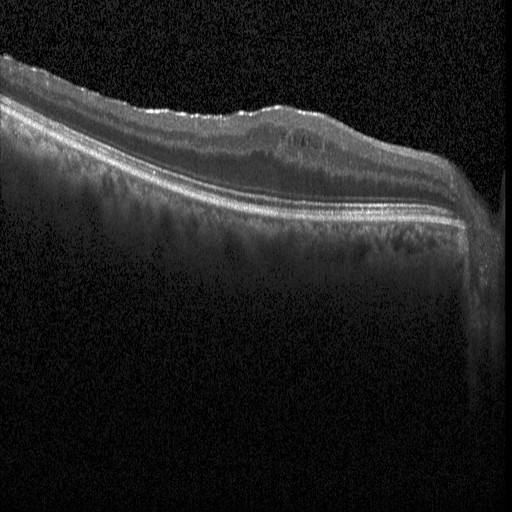 Impression: DME.